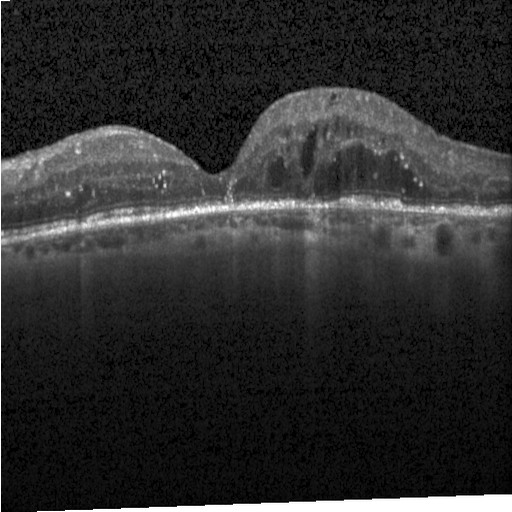

Optical coherence tomography scan · acquired on a Heidelberg Spectralis · spectral-domain optical coherence tomography
DME.